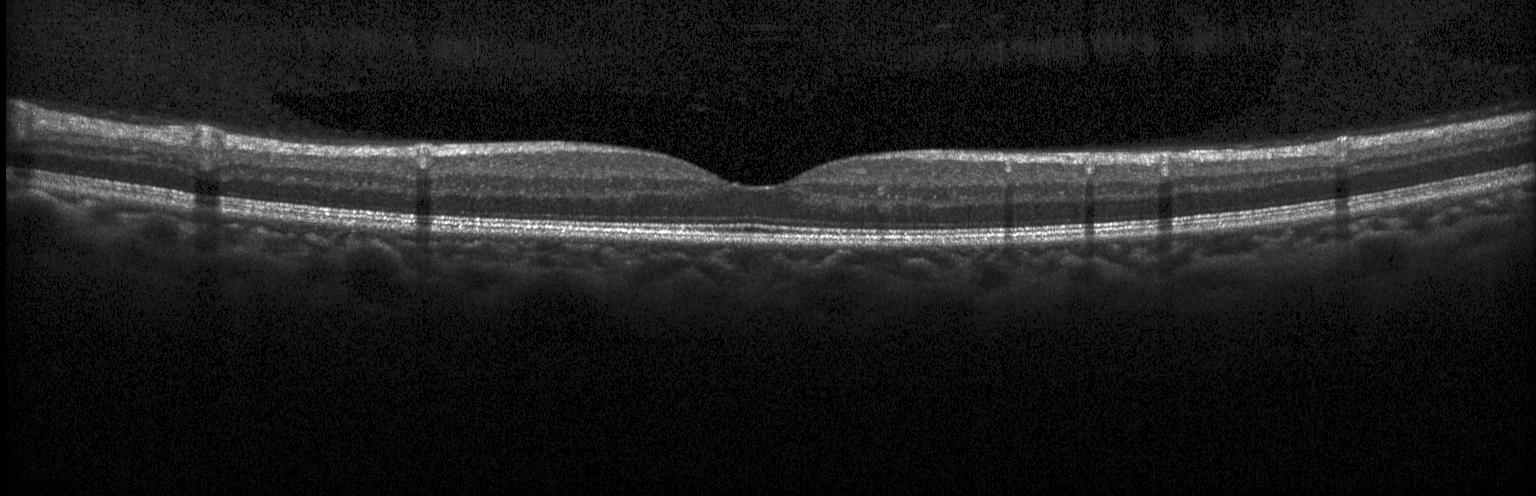 This B-scan demonstrates neither CNV, DME, nor drusen.